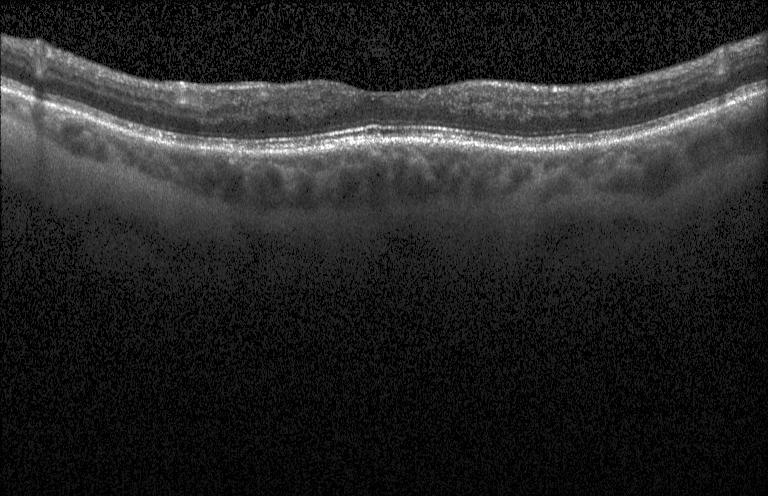

OCT finding: no evidence of CNV, DME, or drusen.